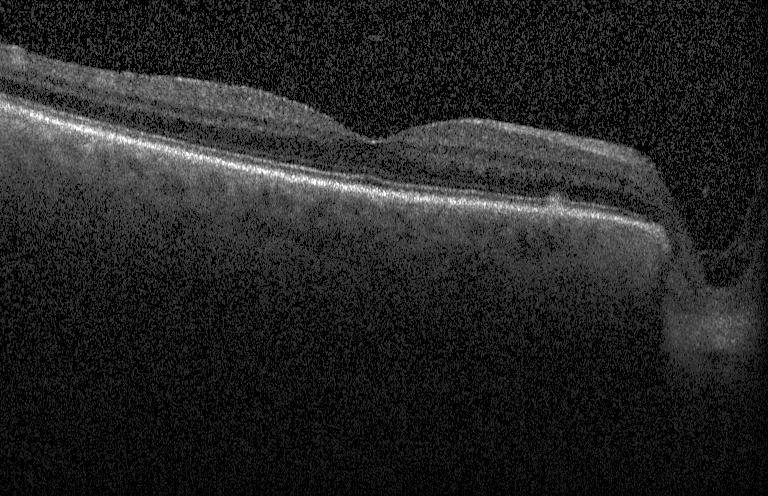

OCT B-scan showing multiple drusen.